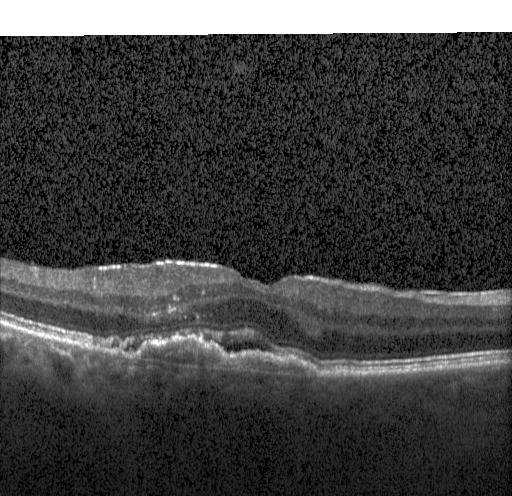

Optical coherence tomography scan. This B-scan demonstrates choroidal neovascularization (CNV).